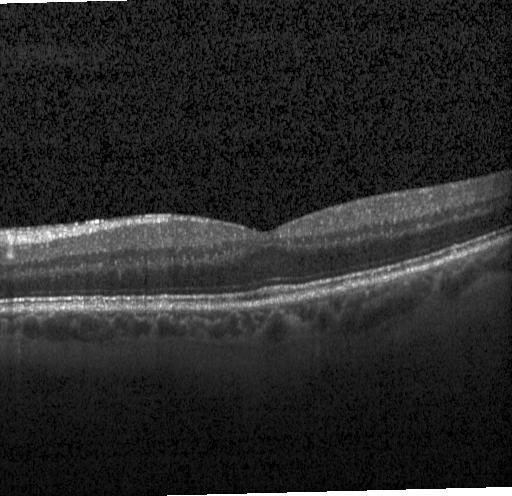

Optical coherence tomography scan · spectral-domain optical coherence tomography.
Impression: no evidence of choroidal neovascularization, diabetic macular edema, or drusen.